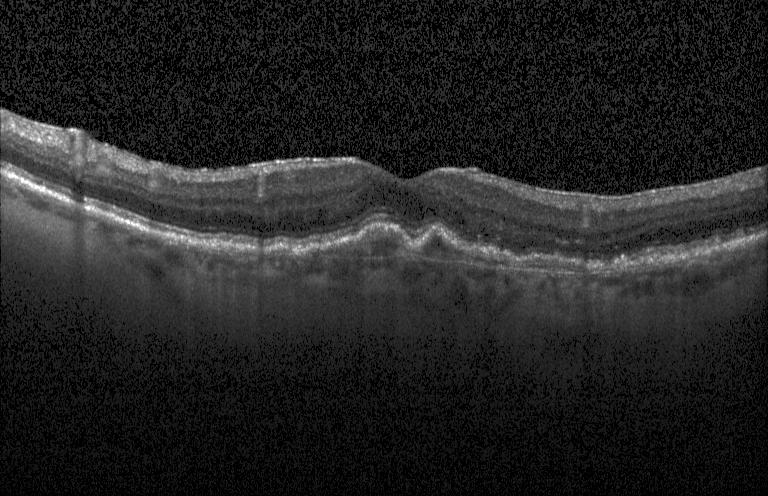 Spectral-domain OCT, OCT line scan — Impression: choroidal neovascularization (CNV).